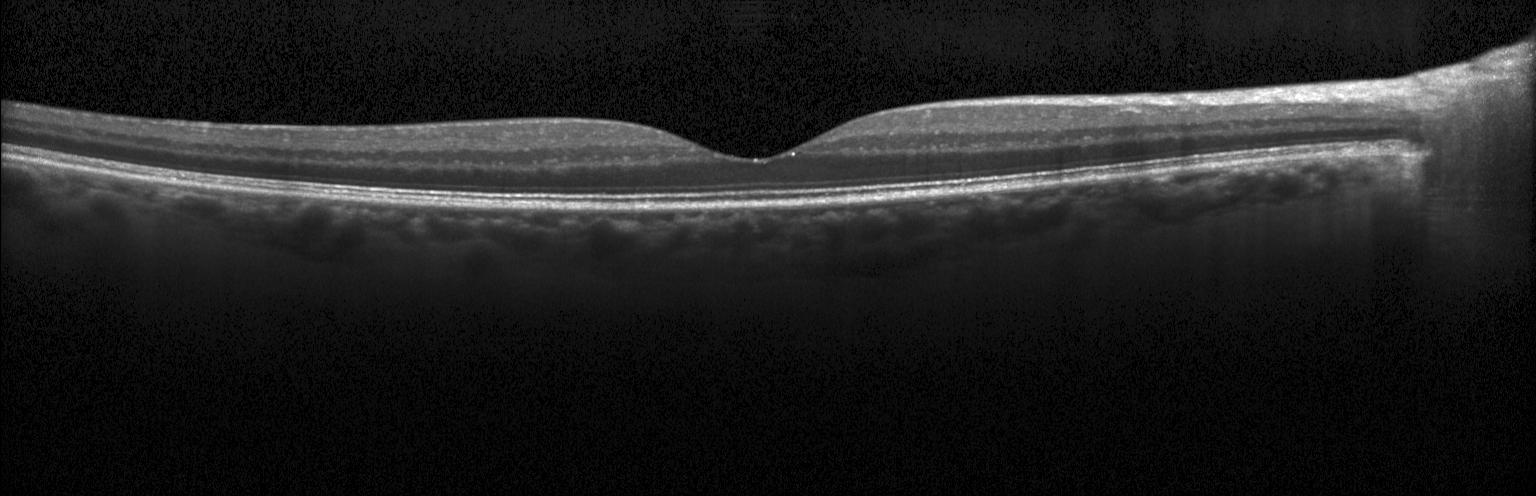

Optical coherence tomography B-scan
Diagnosis: neither choroidal neovascularization, diabetic macular edema, nor drusen.